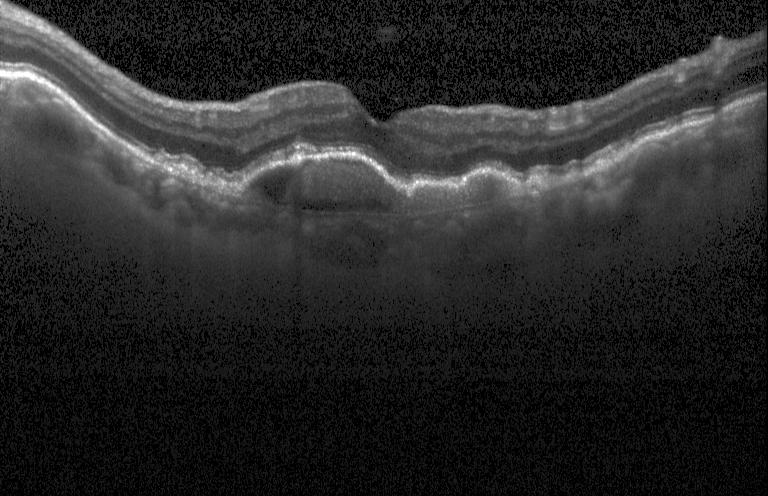 OCT line scan.
Impression: multiple drusen.